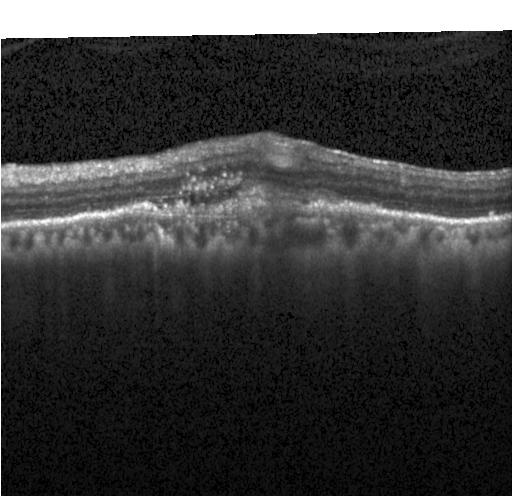
Horizontal scan through the fovea. SD-OCT. Retinal OCT cross-section. Heidelberg Spectralis
Diagnosis: choroidal neovascularization (CNV).